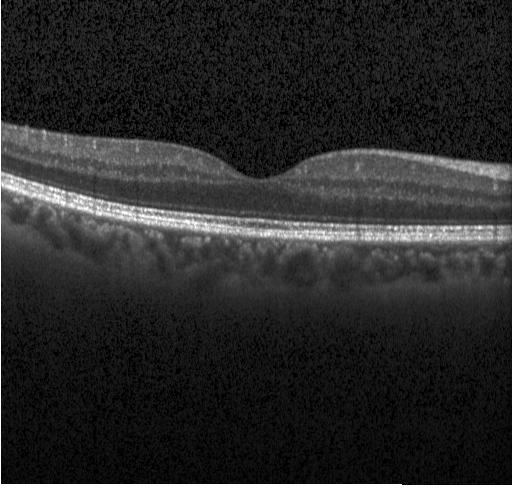

Dx: neither choroidal neovascularization, diabetic macular edema, nor drusen.